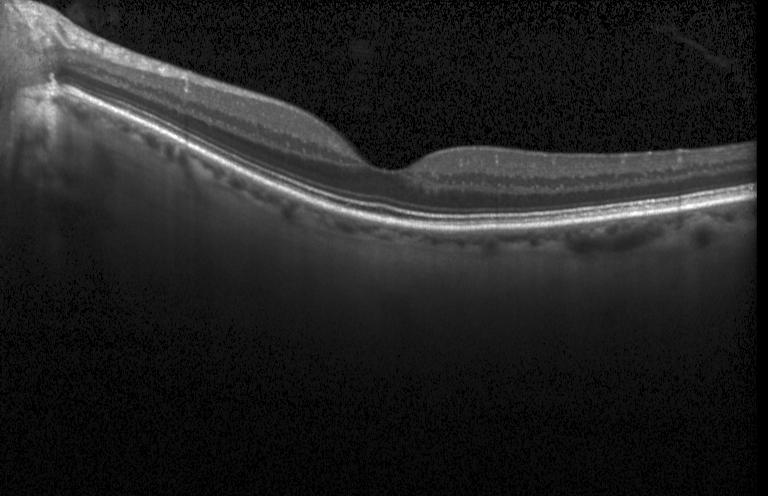
SD-OCT, through the macula, instrument: Heidelberg Spectralis, OCT line scan.
Finding: no choroidal neovascularization, diabetic macular edema, or drusen.